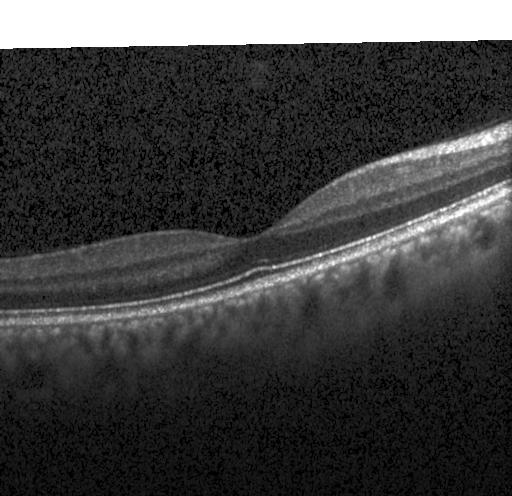 Optical coherence tomography scan.
Dx: no CNV, no DME, and no drusen.